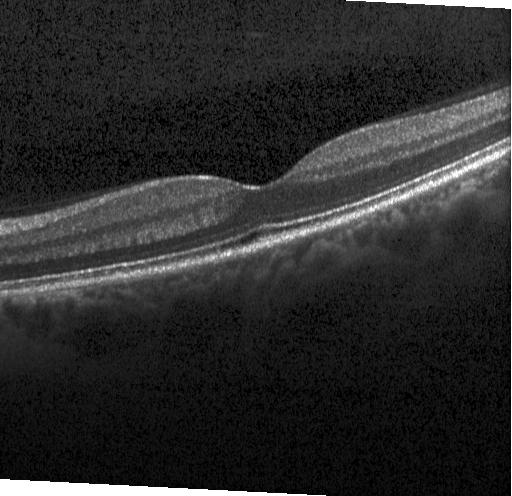

Impression: no choroidal neovascularization, no diabetic macular edema, and no drusen.